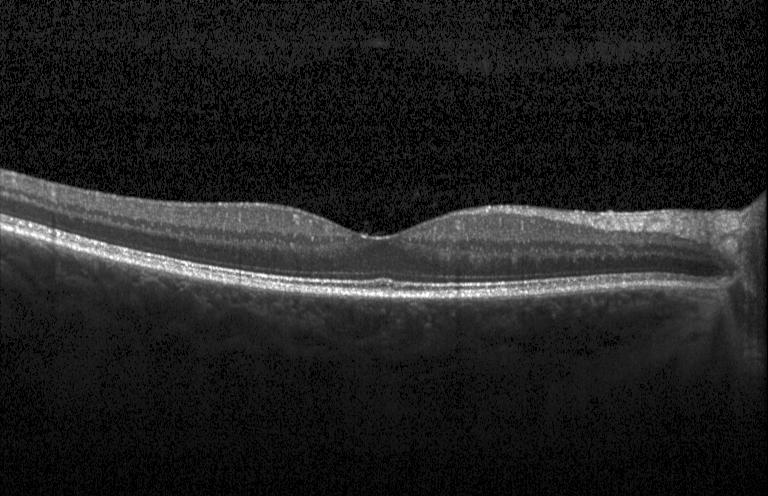 Through the macula; OCT line scan; spectral-domain optical coherence tomography; Heidelberg Spectralis OCT system. Impression: no choroidal neovascularization, diabetic macular edema, or drusen.